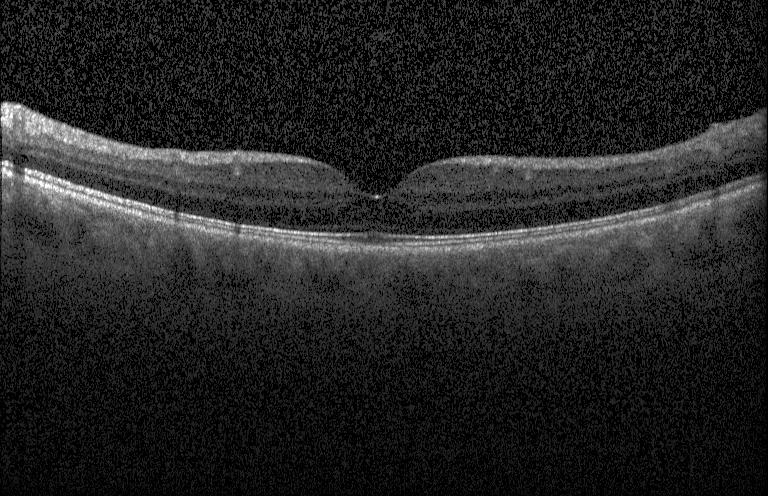

Finding: neither choroidal neovascularization, diabetic macular edema, nor drusen.